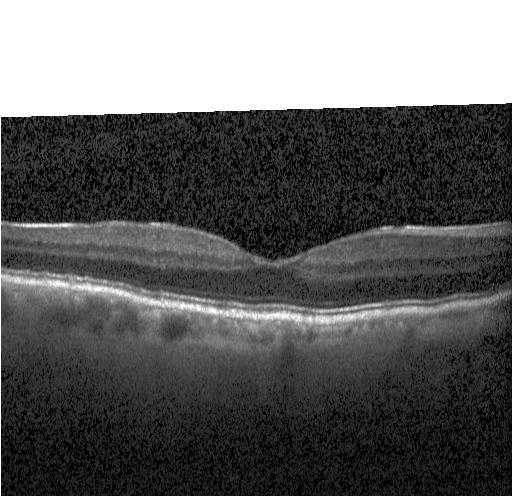 Macular OCT demonstrating no choroidal neovascularization, no diabetic macular edema, and no drusen.